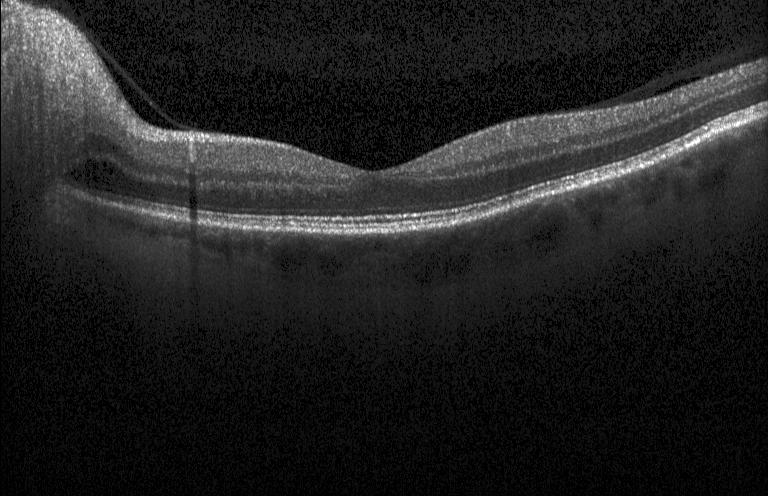 Retinal OCT B-scan · instrument: Heidelberg Spectralis · fovea-centered.
Impression: no evidence of choroidal neovascularization, diabetic macular edema, or drusen.